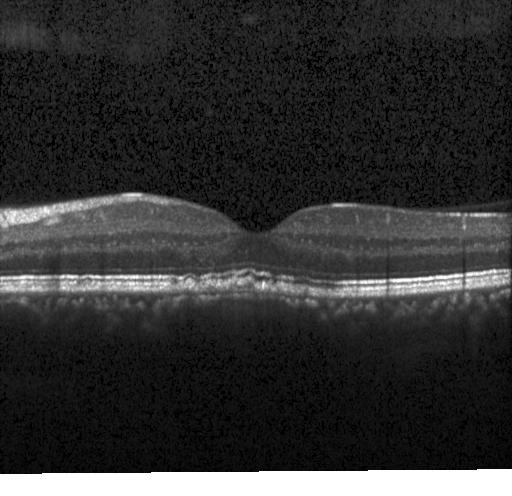 Retinal OCT B-scan. Heidelberg Spectralis. Spectral-domain OCT.
Diagnosis: drusen.